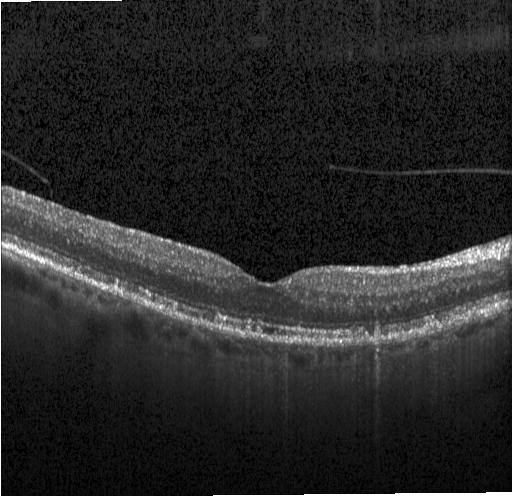 OCT scan showing sub-RPE drusenoid deposits.